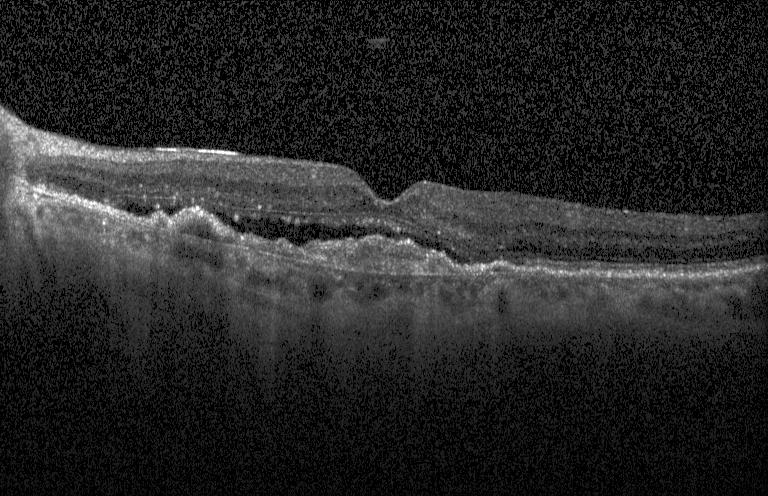
The scan shows a choroidal neovascular membrane.